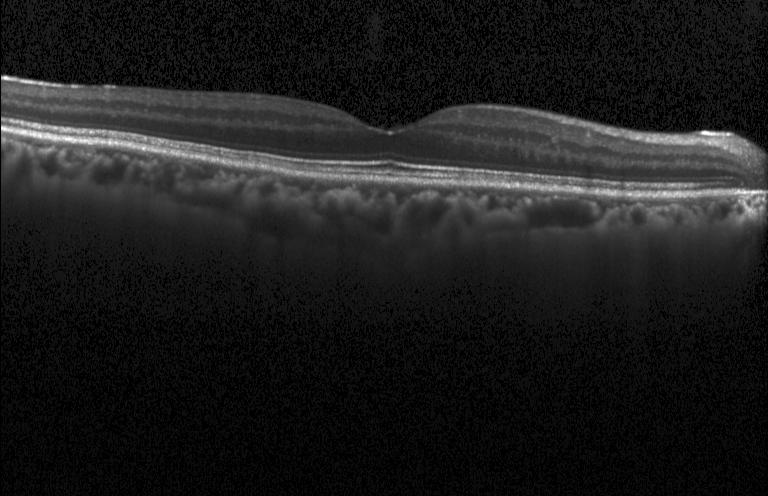 Optical coherence tomography scan · Heidelberg Spectralis · spectral-domain optical coherence tomography · fovea-centered — The scan shows neither choroidal neovascularization, diabetic macular edema, nor drusen.